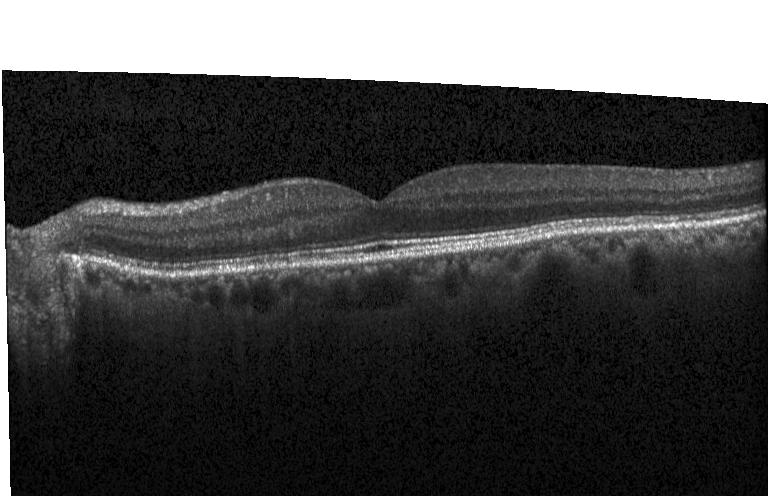

OCT finding: no evidence of choroidal neovascularization, diabetic macular edema, or drusen.